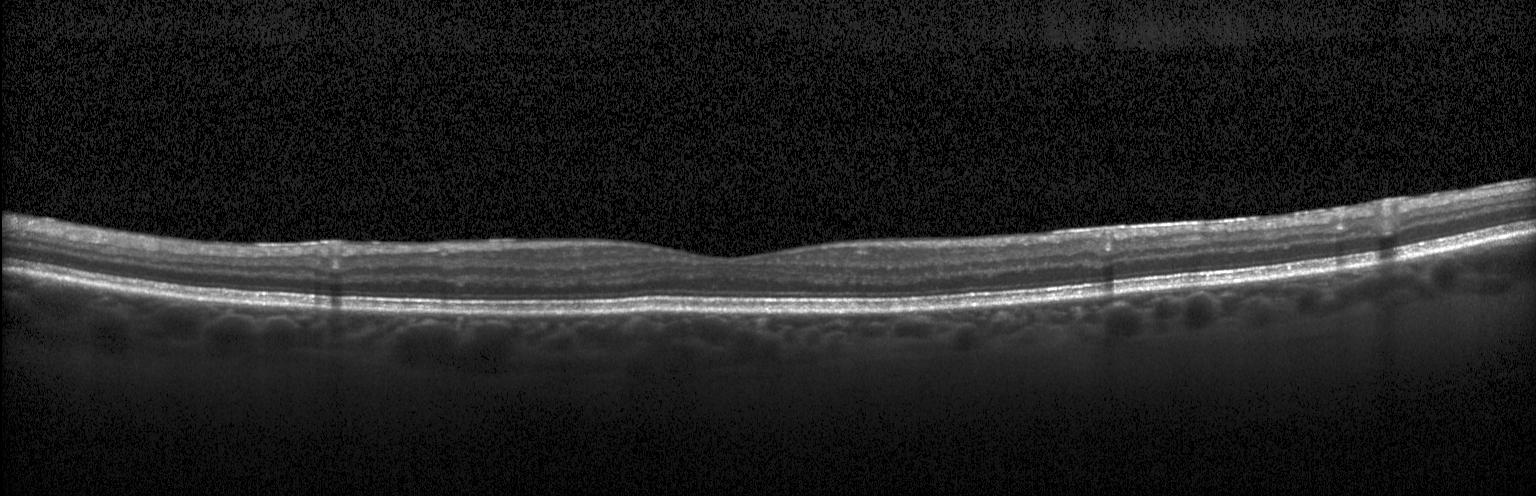

This B-scan demonstrates neither choroidal neovascularization, diabetic macular edema, nor drusen.